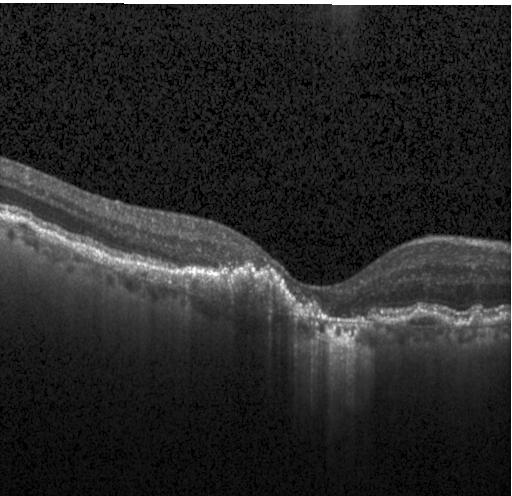
Heidelberg Spectralis; spectral-domain optical coherence tomography; retinal OCT B-scan; through the macula. Impression: a choroidal neovascular membrane.